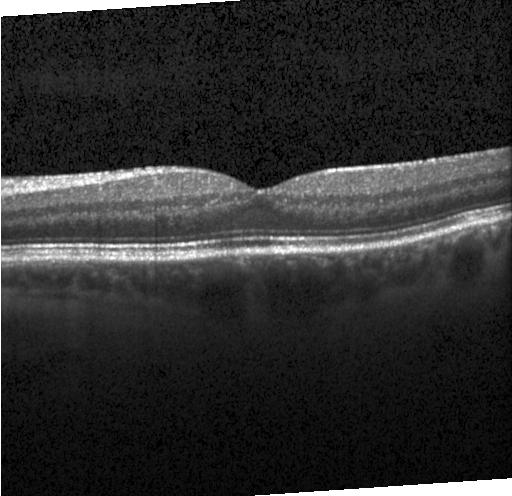 Impression: no evidence of choroidal neovascularization, diabetic macular edema, or drusen.